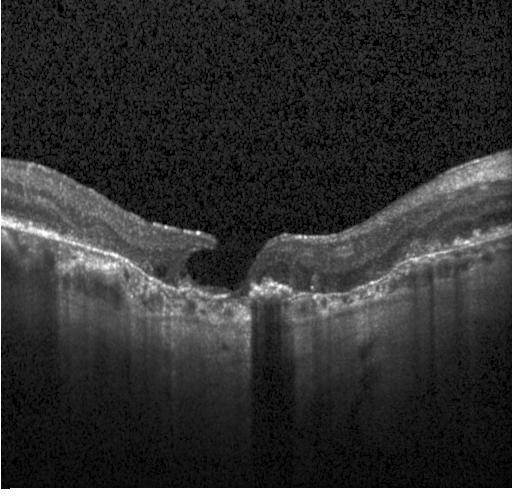 A choroidal neovascular membrane.